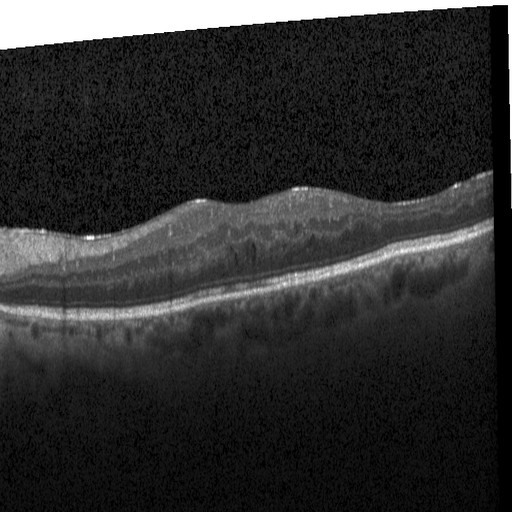

This B-scan demonstrates diabetic macular edema.